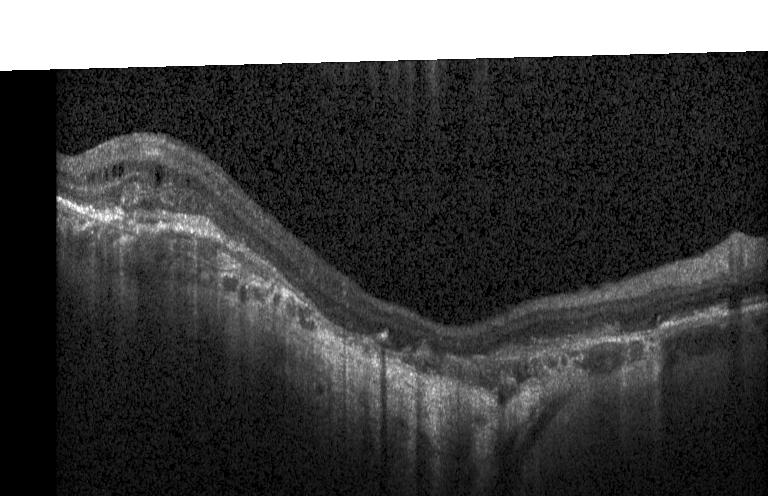

Optical coherence tomography scan.
This B-scan demonstrates a choroidal neovascular membrane.